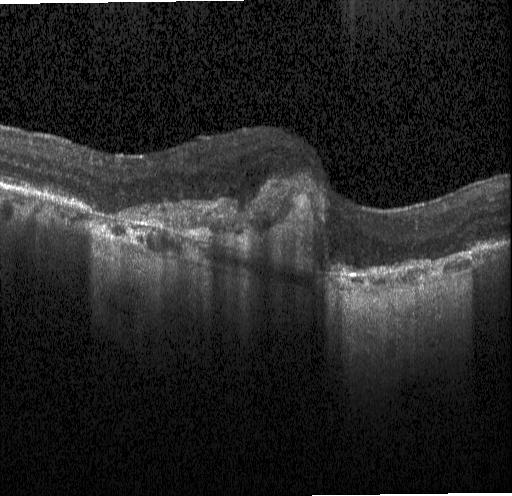 Assessment: CNV.